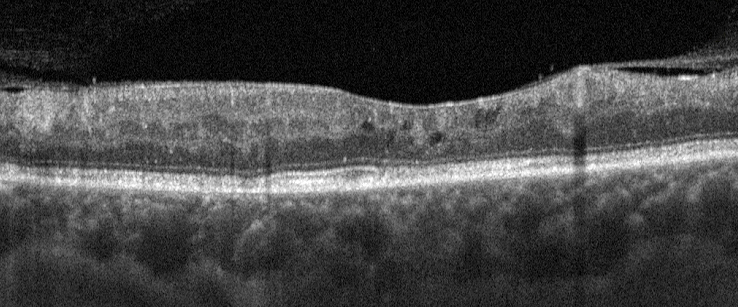
Instrument: Optovue Avanti RTVue XR · optical coherence tomography scan · through the macula. Diabetic macular edema (DME).